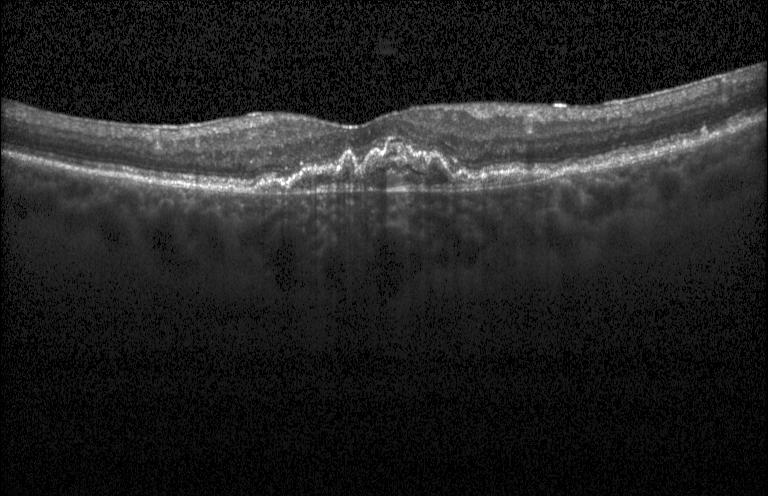
Optical coherence tomography scan. Spectral-domain optical coherence tomography. OCT finding: a choroidal neovascular membrane.